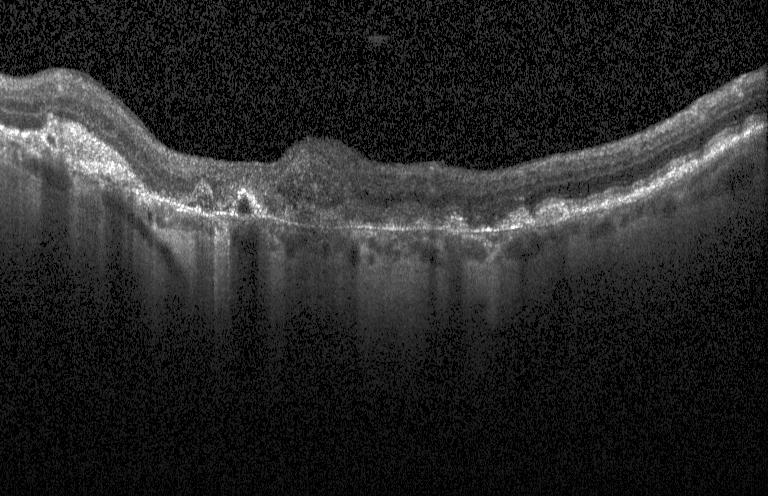
OCT B-scan showing a choroidal neovascular membrane.